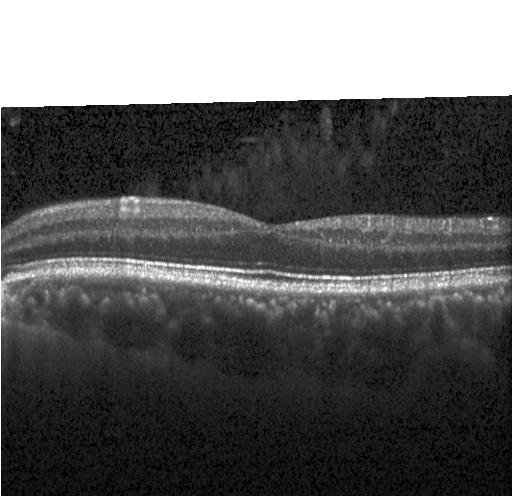
The scan shows no evidence of choroidal neovascularization, diabetic macular edema, or drusen.